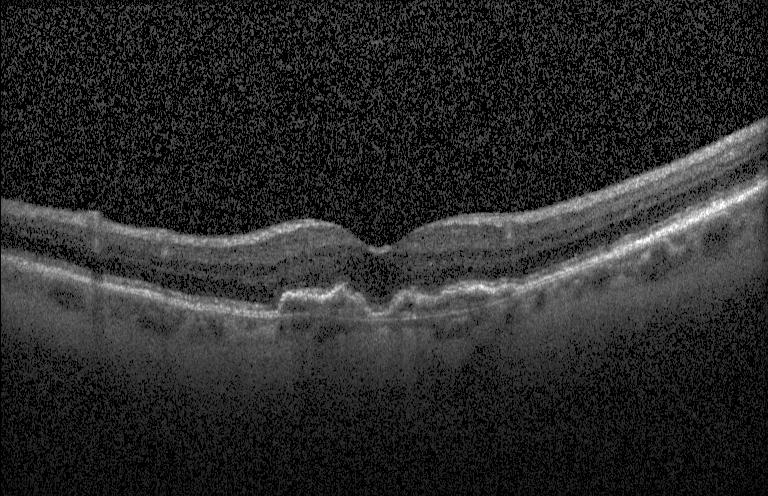

Retinal OCT cross-section — Macular OCT: CNV.